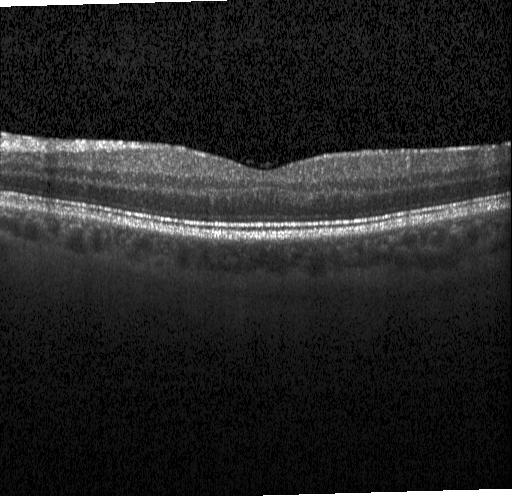

OCT line scan.
Finding: no choroidal neovascularization, no diabetic macular edema, and no drusen.